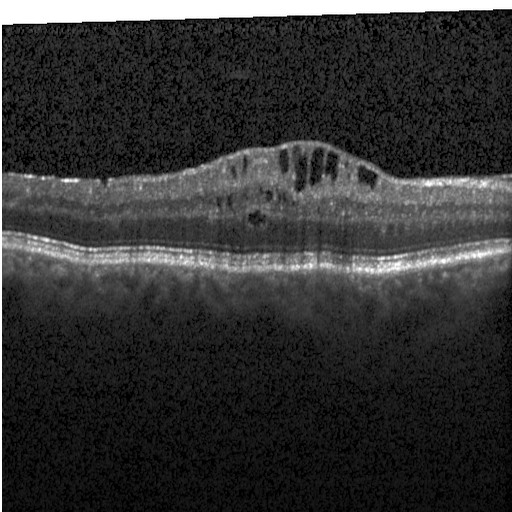
Heidelberg Spectralis, centered on the fovea, optical coherence tomography B-scan — Impression: diabetic macular edema.